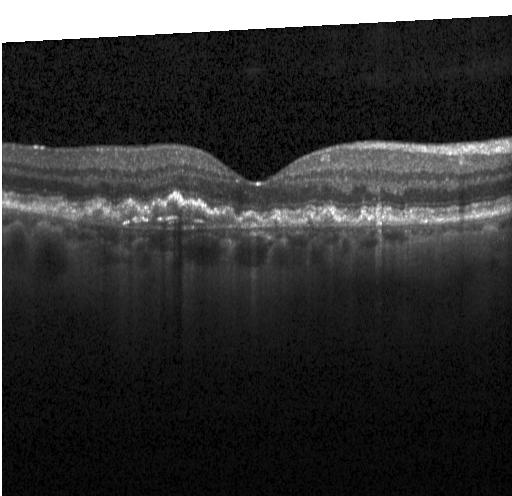

SD-OCT. Optical coherence tomography B-scan
OCT finding: a choroidal neovascular membrane.